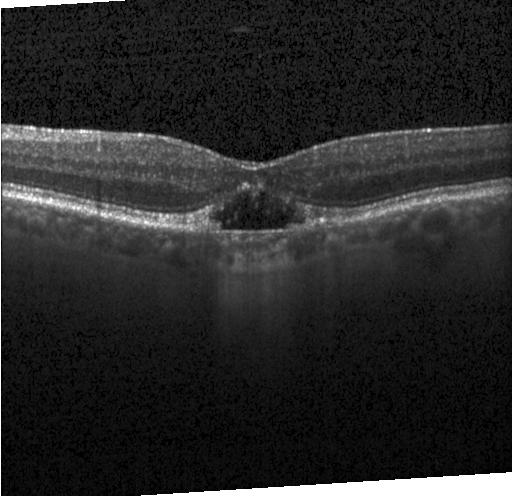
Impression: choroidal neovascularization.